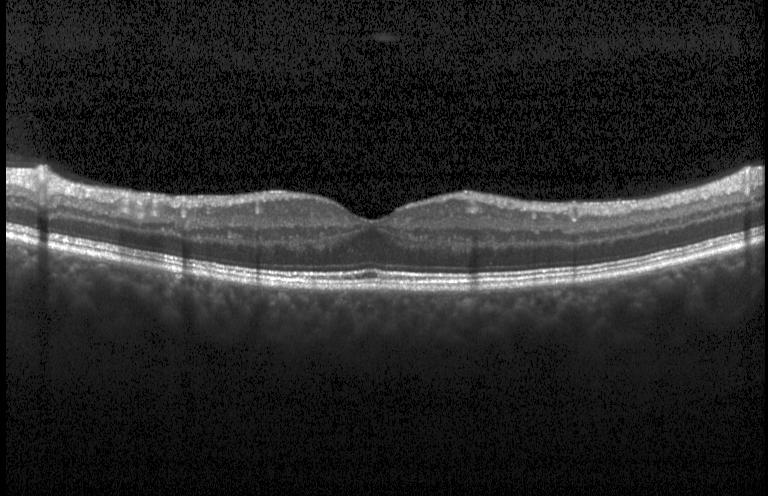
Diagnosis: no evidence of CNV, DME, or drusen.